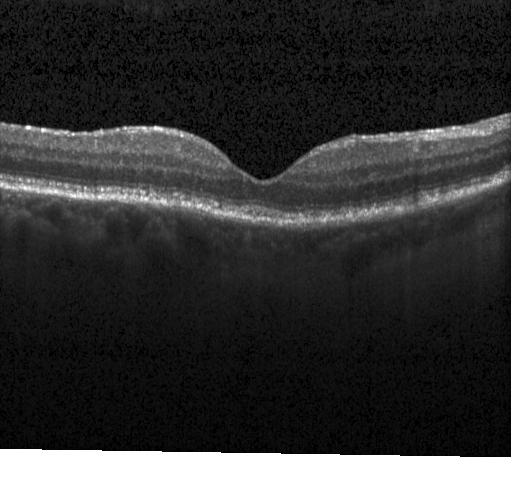
Optical coherence tomography B-scan; Heidelberg Spectralis; spectral-domain OCT. Diagnosis: no evidence of CNV, DME, or drusen.